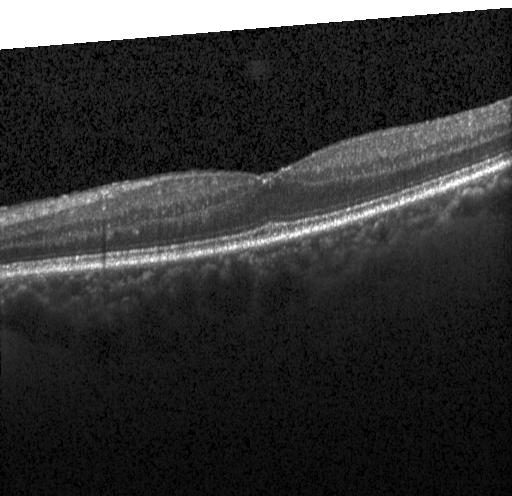 Acquired on a Heidelberg Spectralis · retinal OCT cross-section
Finding: no choroidal neovascularization, no diabetic macular edema, and no drusen.